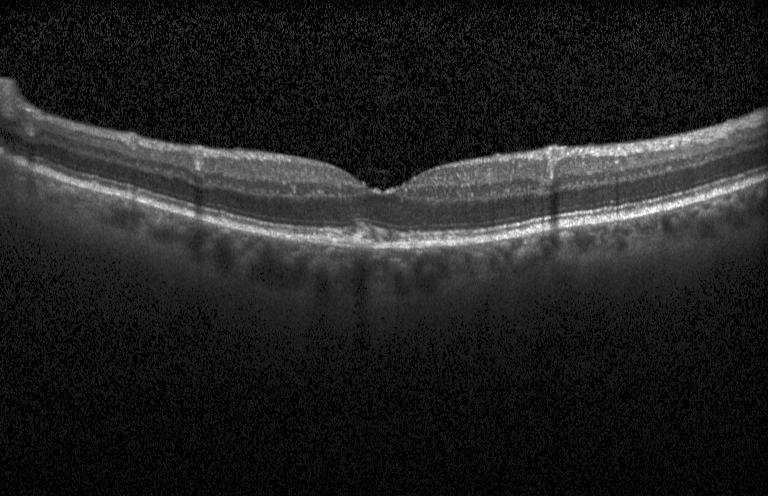 OCT B-scan showing sub-RPE drusenoid deposits.